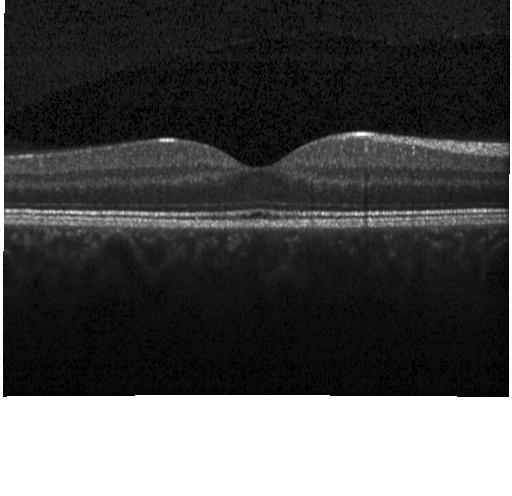 Acquired on a Heidelberg Spectralis. OCT line scan. Horizontal scan through the fovea. Spectral-domain optical coherence tomography. Diagnosis: no CNV, no DME, and no drusen.